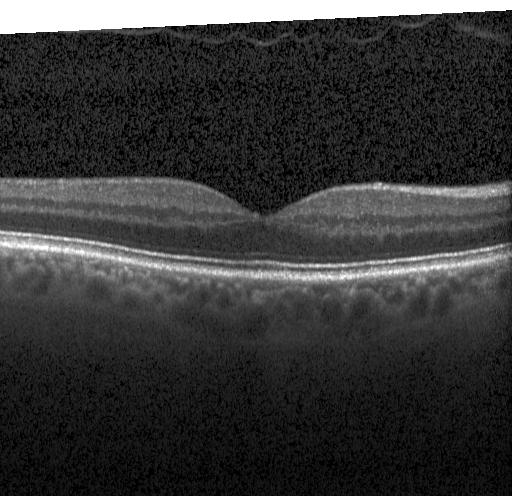

OCT finding: no evidence of choroidal neovascularization, diabetic macular edema, or drusen.